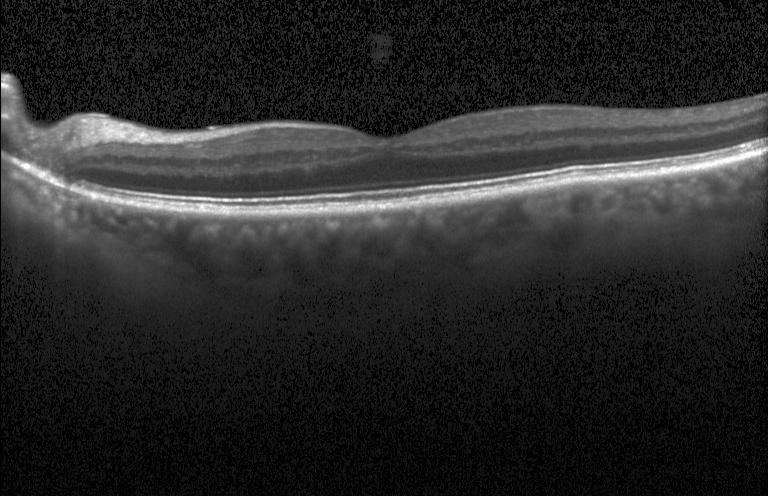

OCT B-scan, acquired on a Heidelberg Spectralis, centered on the fovea, spectral-domain OCT. Impression: no choroidal neovascularization, no diabetic macular edema, and no drusen.